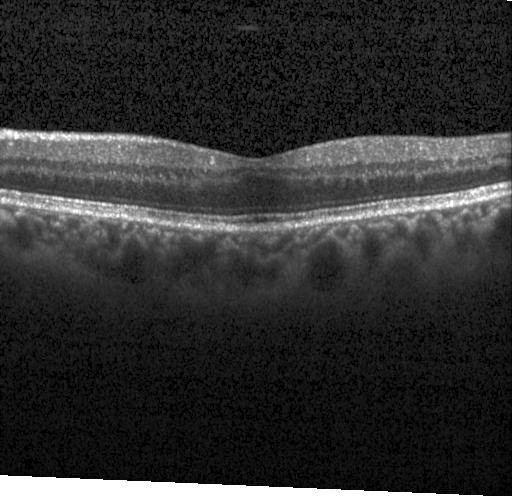
Optical coherence tomography B-scan. Finding: neither CNV, DME, nor drusen.